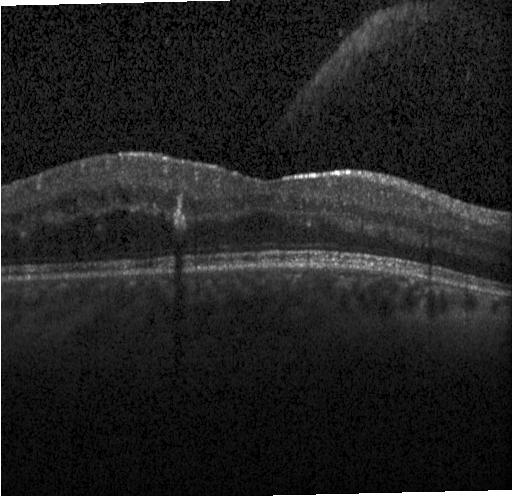
Horizontal scan through the fovea, spectral-domain OCT, optical coherence tomography B-scan
Impression: diabetic macular edema (DME).